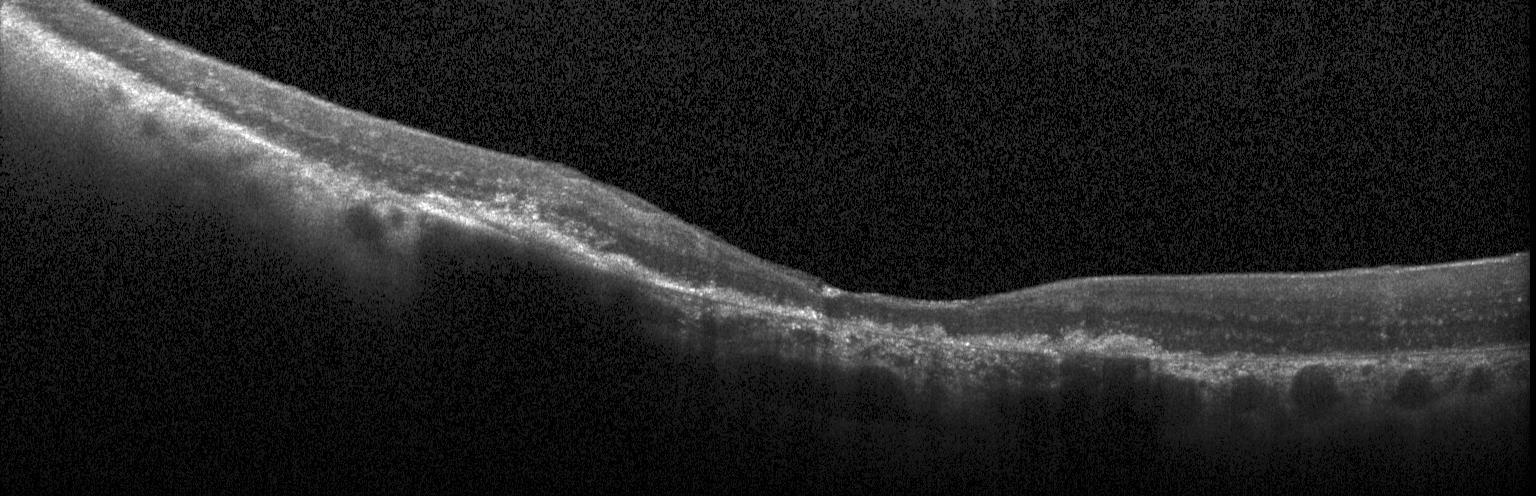

OCT B-scan. OCT finding: CNV.